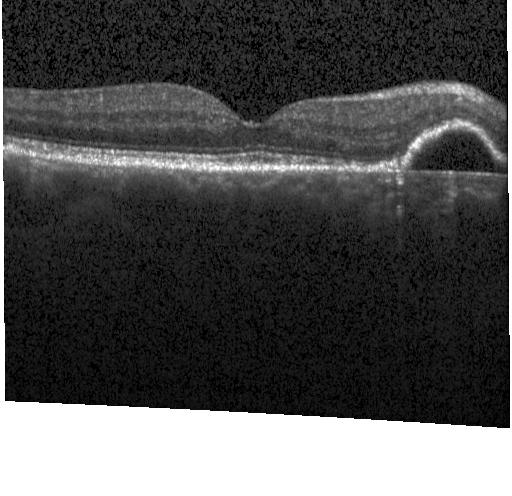
Retinal OCT B-scan — Finding: choroidal neovascularization (CNV).